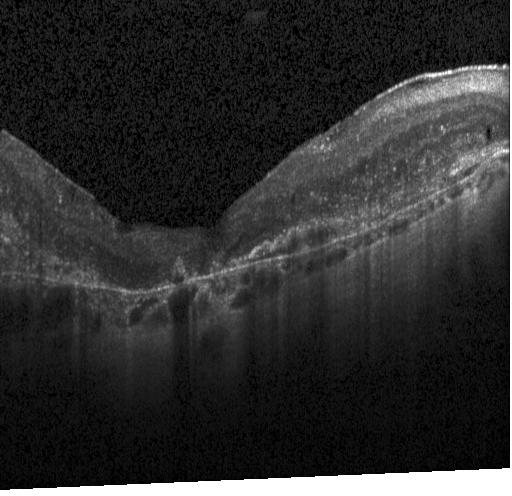

Optical coherence tomography scan.
This B-scan demonstrates a choroidal neovascular membrane.